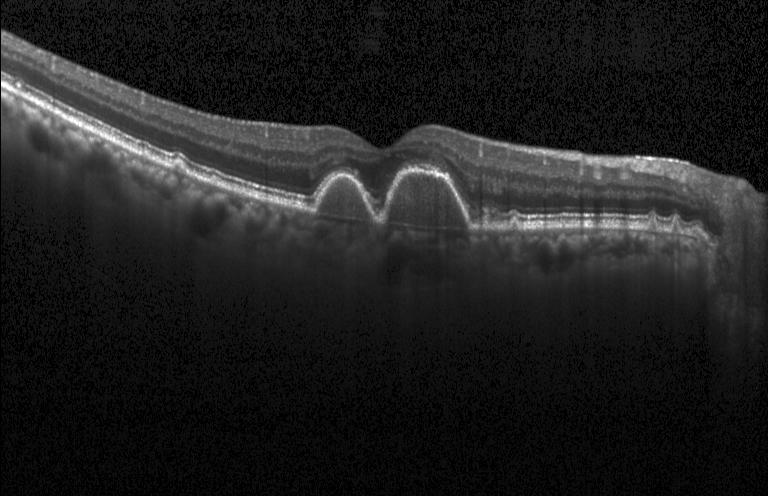
Acquired on a Heidelberg Spectralis · spectral-domain OCT · macular scan · retinal OCT cross-section
Impression: sub-RPE drusenoid deposits.